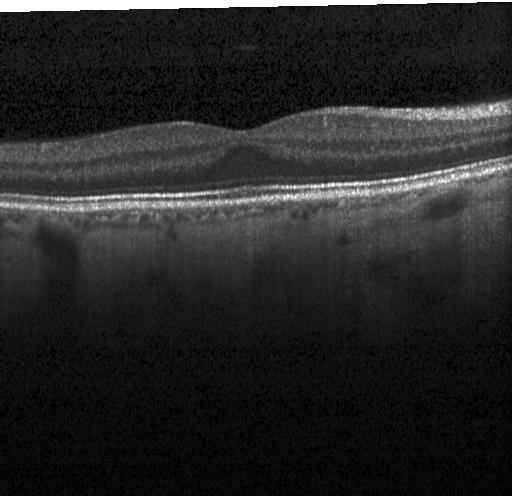 No evidence of choroidal neovascularization, diabetic macular edema, or drusen.